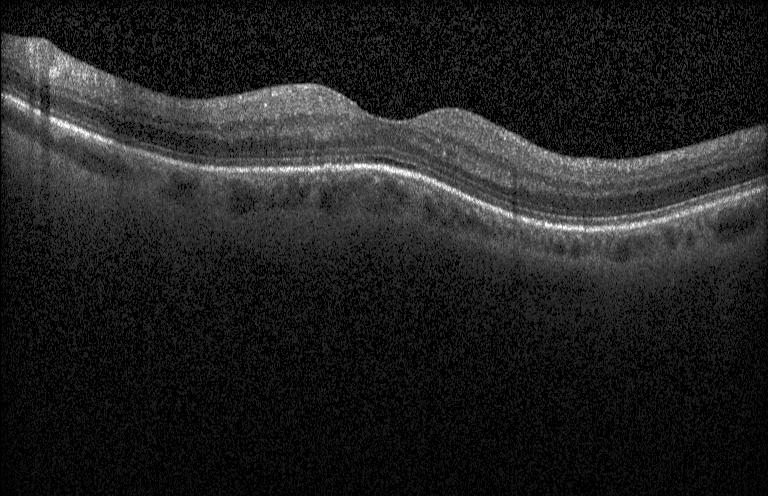
The scan shows no evidence of choroidal neovascularization, diabetic macular edema, or drusen.